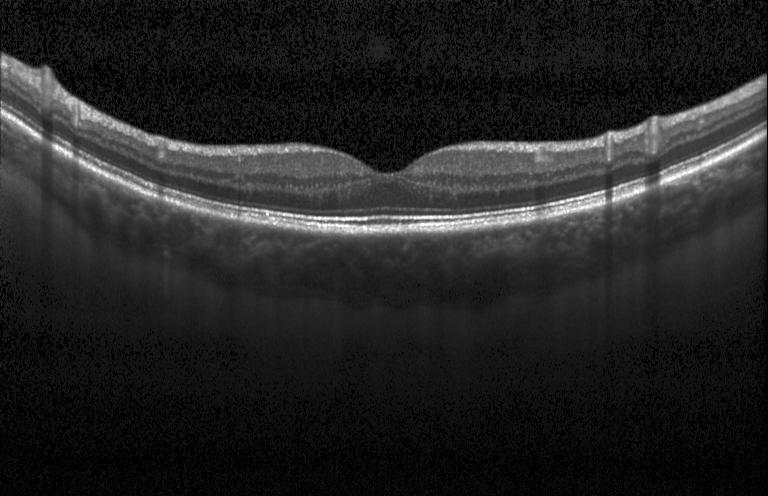
Retinal OCT B-scan. This B-scan demonstrates no choroidal neovascularization, no diabetic macular edema, and no drusen.